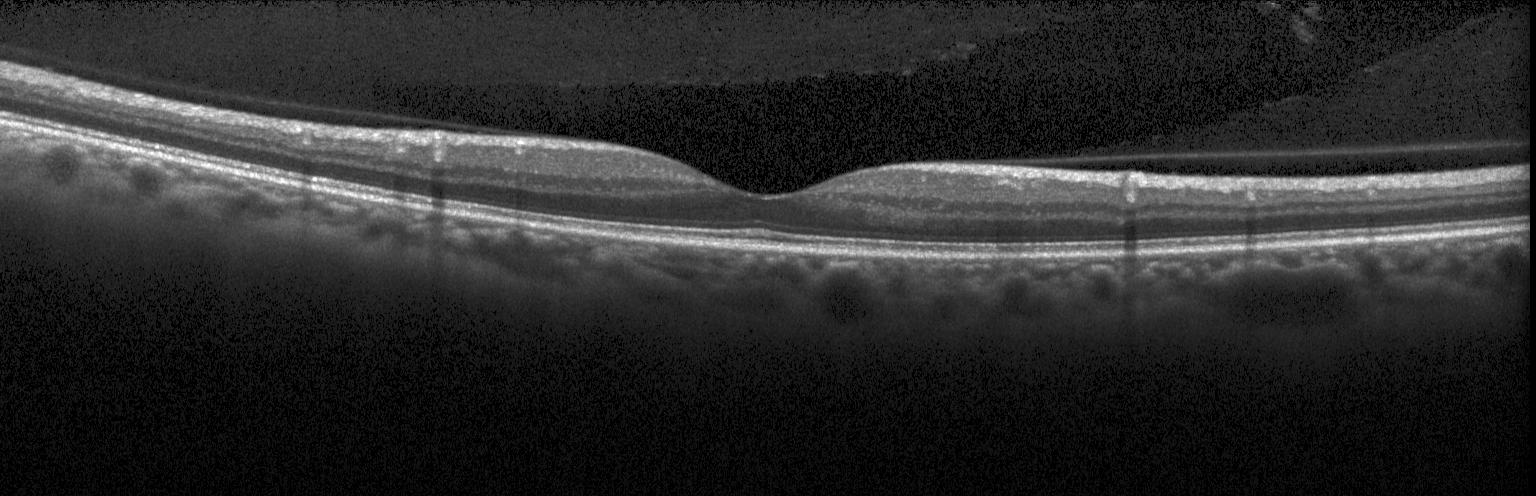
Through the macula, OCT line scan, acquired on a Heidelberg Spectralis. Finding: no evidence of CNV, DME, or drusen.